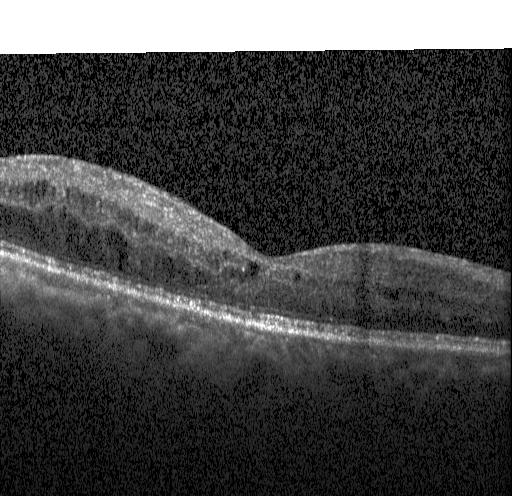

Finding: diabetic macular edema (DME).